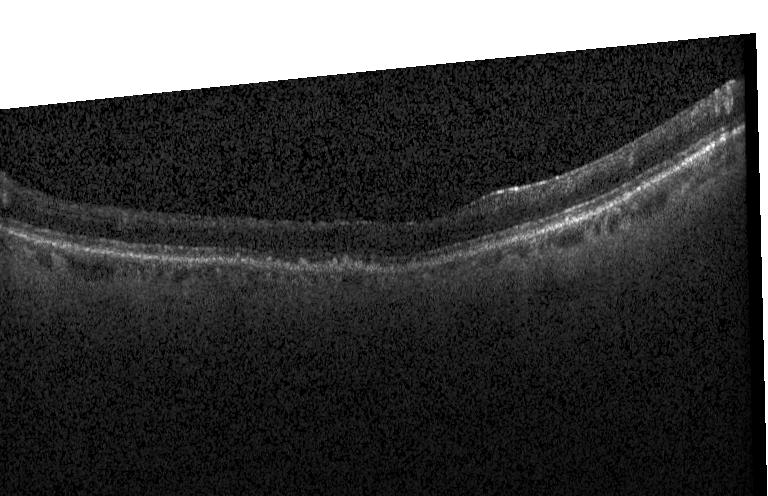
Optical coherence tomography scan · Heidelberg Spectralis · spectral-domain optical coherence tomography · through the macula
Assessment: sub-RPE drusenoid deposits.